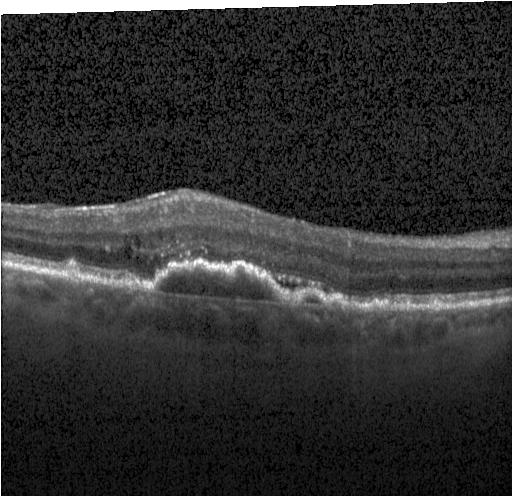
Diagnosis: a choroidal neovascular membrane.